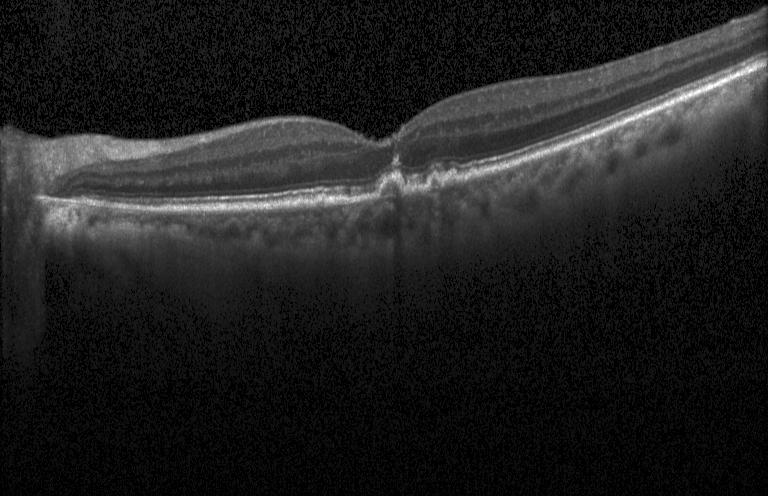 Sub-RPE drusenoid deposits.